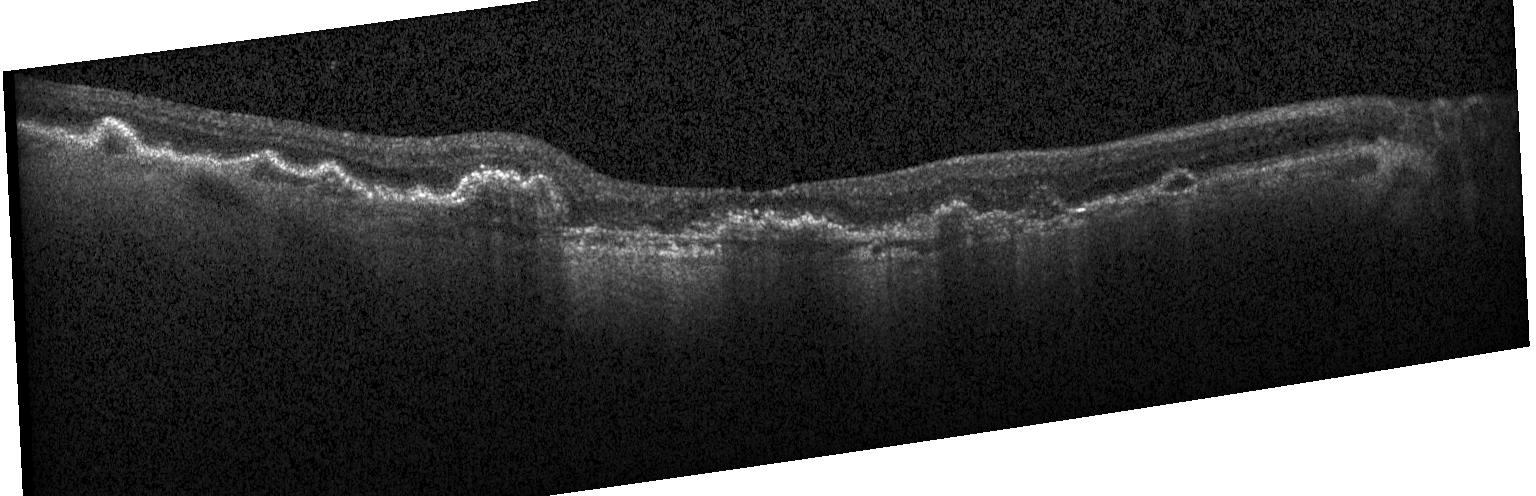

Through the macula, optical coherence tomography B-scan, spectral-domain optical coherence tomography. Diagnosis: choroidal neovascularization (CNV).